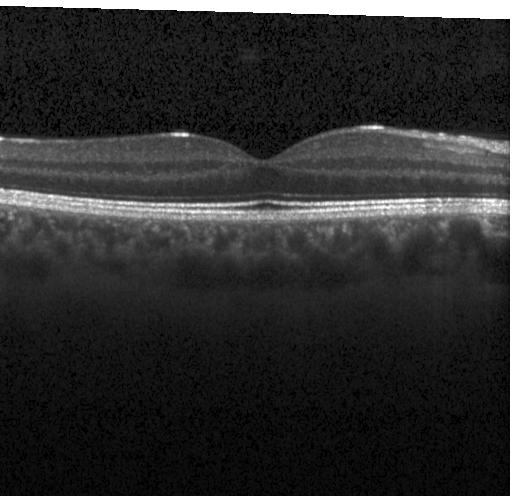
Centered on the fovea; spectral-domain optical coherence tomography; Heidelberg Spectralis; retinal OCT B-scan
Finding: neither choroidal neovascularization, diabetic macular edema, nor drusen.